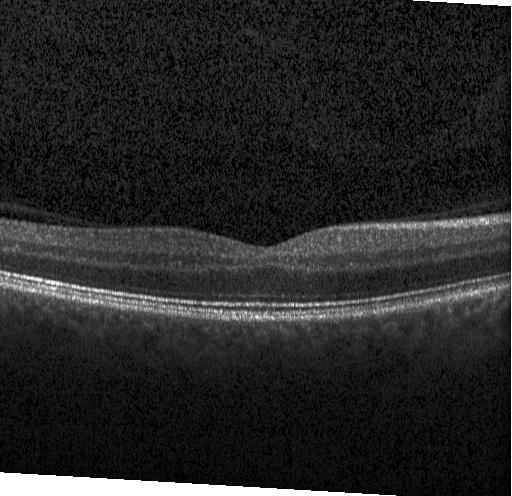
OCT finding: no evidence of choroidal neovascularization, diabetic macular edema, or drusen.